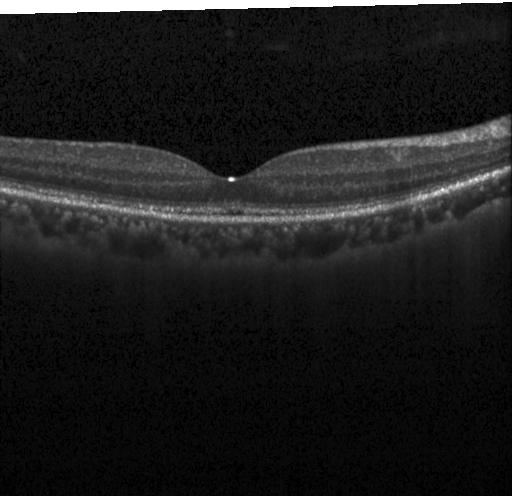
OCT line scan. This B-scan demonstrates neither CNV, DME, nor drusen.